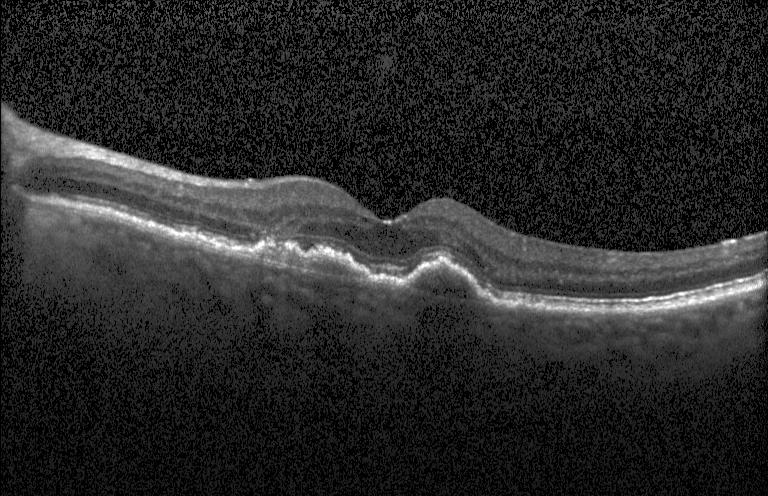

OCT line scan.
A choroidal neovascular membrane.